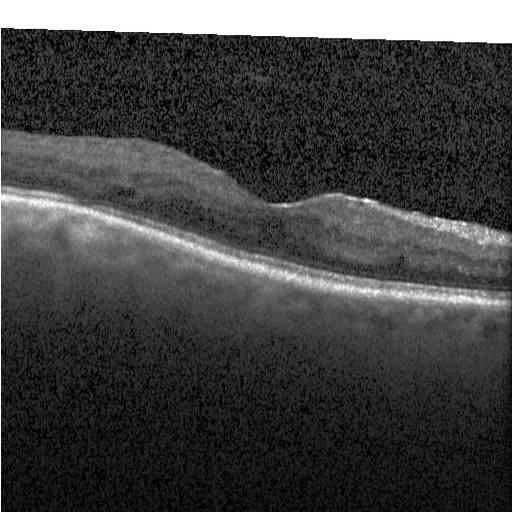 Spectral-domain OCT · instrument: Heidelberg Spectralis · optical coherence tomography B-scan · fovea-centered.
Macular OCT: DME.